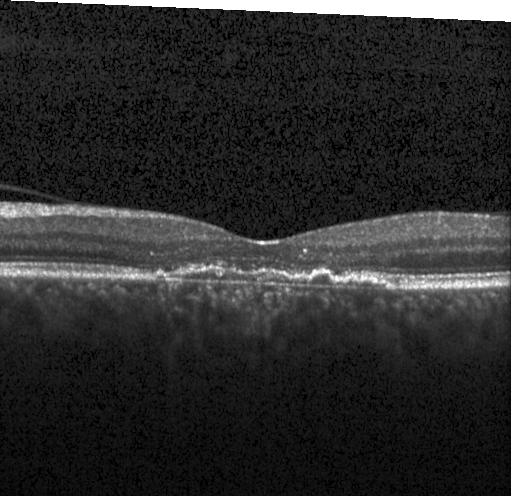 Heidelberg Spectralis. OCT line scan
Dx: a choroidal neovascular membrane.